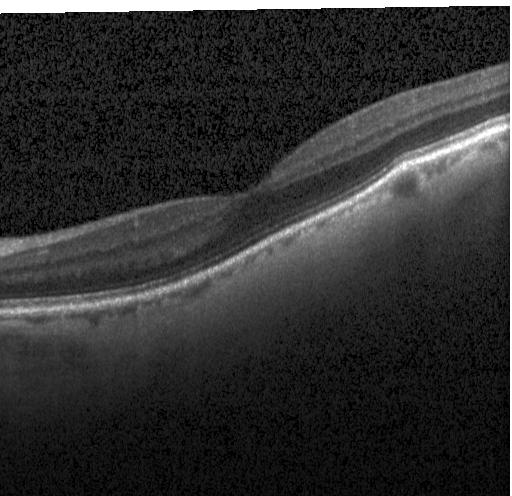

Optical coherence tomography scan; spectral-domain OCT; acquired on a Heidelberg Spectralis — Finding: neither CNV, DME, nor drusen.